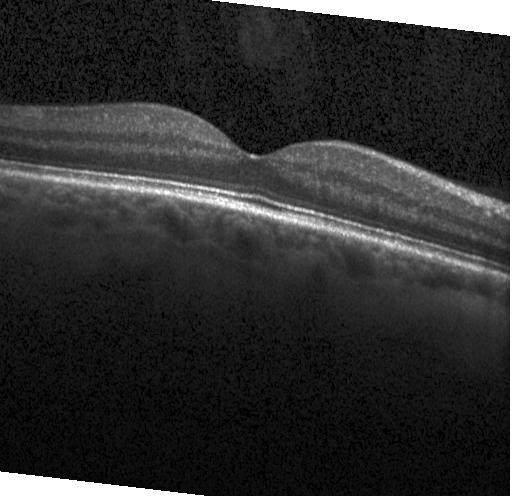 Optical coherence tomography B-scan · Heidelberg Spectralis
Diagnosis: no choroidal neovascularization, no diabetic macular edema, and no drusen.